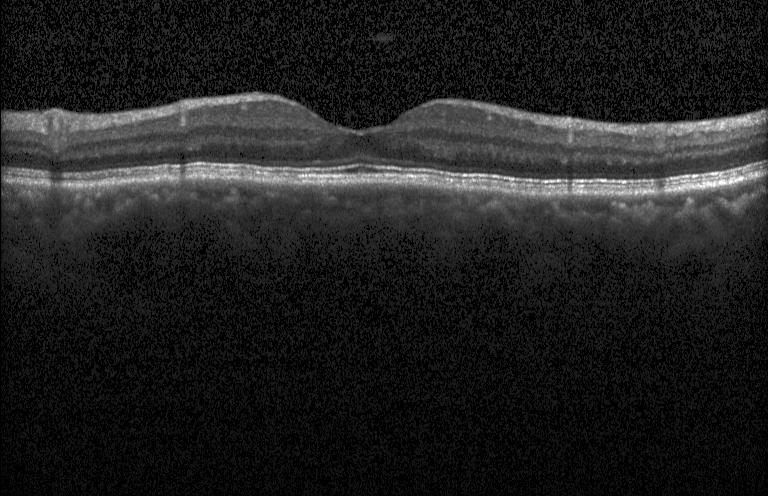

Spectral-domain optical coherence tomography; OCT B-scan. The scan shows no CNV, DME, or drusen.